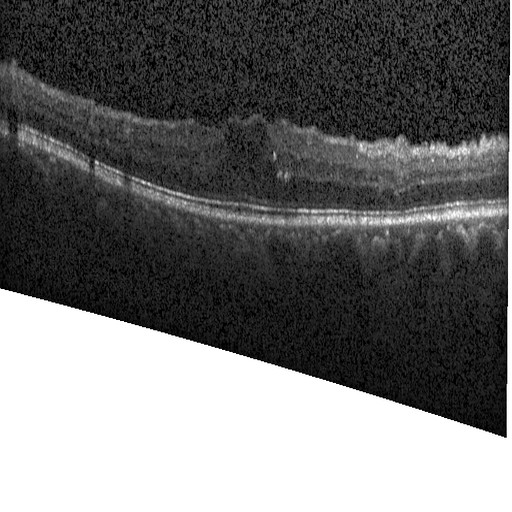

Spectral-domain optical coherence tomography; OCT B-scan; fovea-centered; acquired on a Heidelberg Spectralis.
Finding: DME.